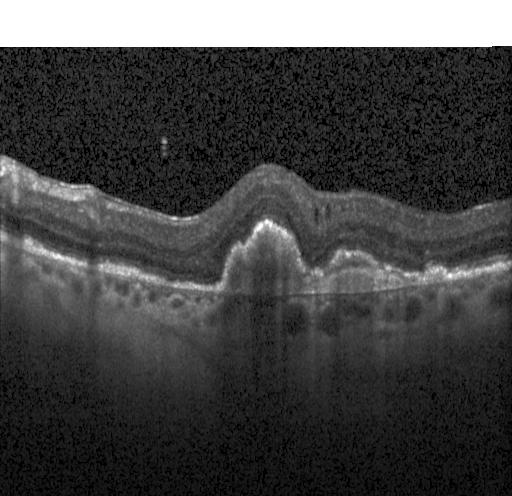 OCT line scan.
Assessment: CNV.